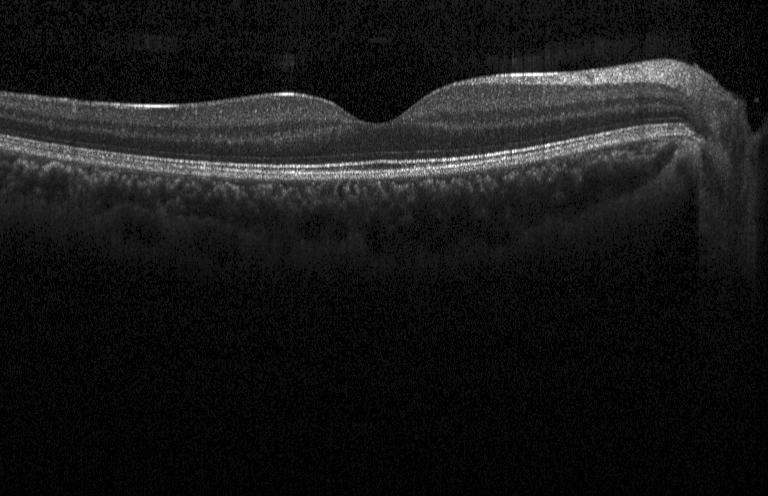
Spectral-domain optical coherence tomography; acquired on a Heidelberg Spectralis; retinal OCT cross-section.
Macular OCT: neither choroidal neovascularization, diabetic macular edema, nor drusen.